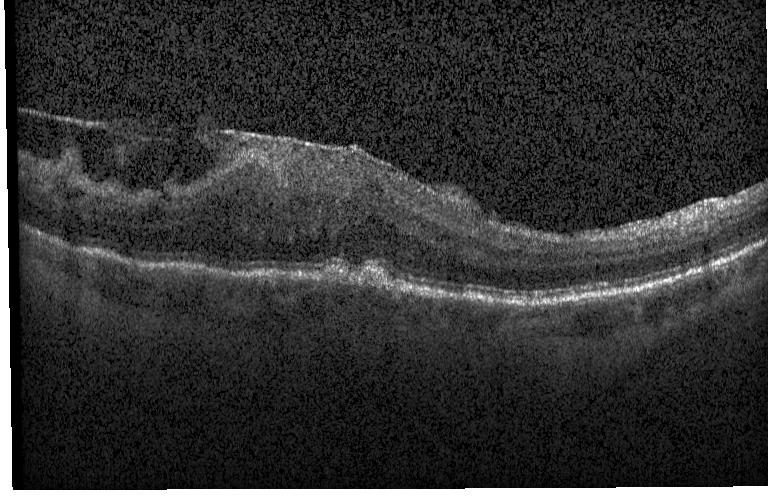 Retinal OCT cross-section showing drusen.